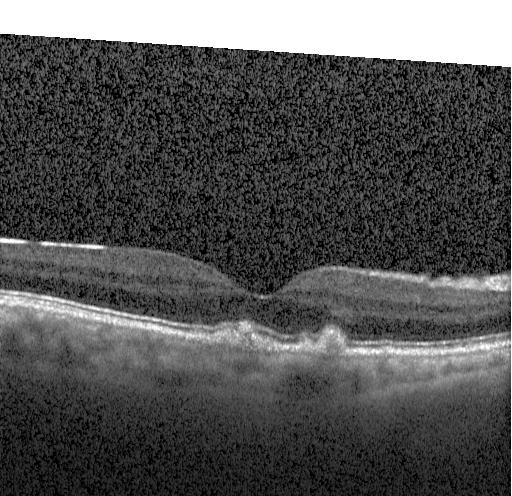

Retinal OCT cross-section — Multiple drusen.